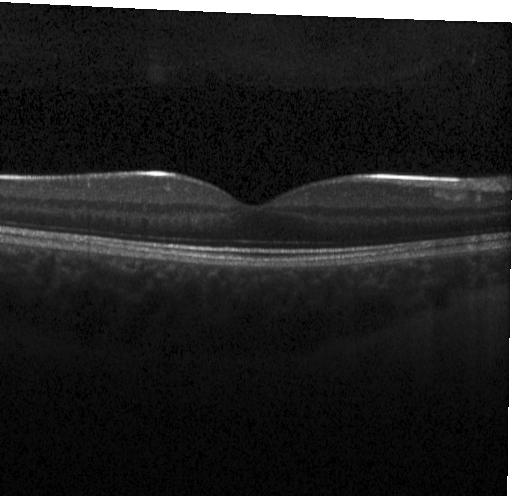 Spectral-domain OCT, OCT B-scan, through the macula, instrument: Heidelberg Spectralis. This B-scan demonstrates no evidence of choroidal neovascularization, diabetic macular edema, or drusen.